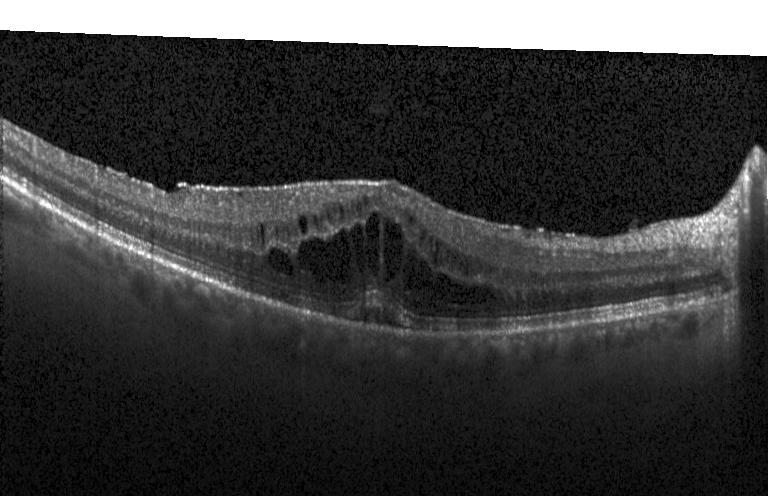
Finding: diabetic macular edema.